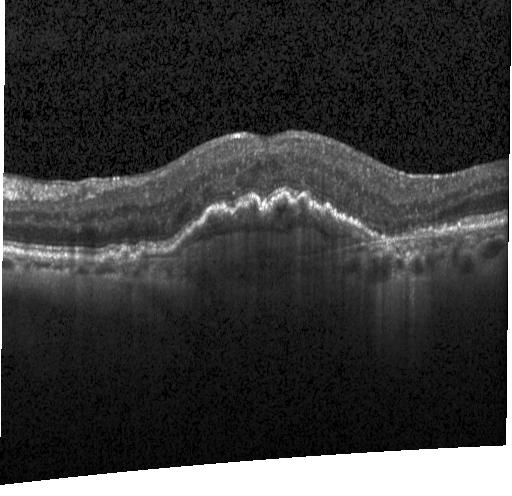

Macular scan · Heidelberg Spectralis OCT system · optical coherence tomography B-scan · SD-OCT. A choroidal neovascular membrane.